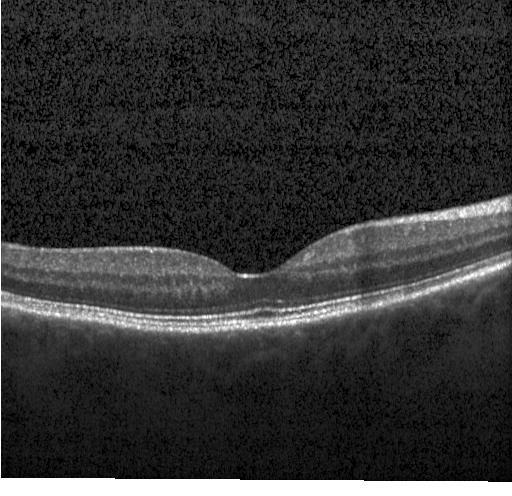

Fovea-centered, retinal OCT B-scan, spectral-domain optical coherence tomography
Assessment: neither CNV, DME, nor drusen.